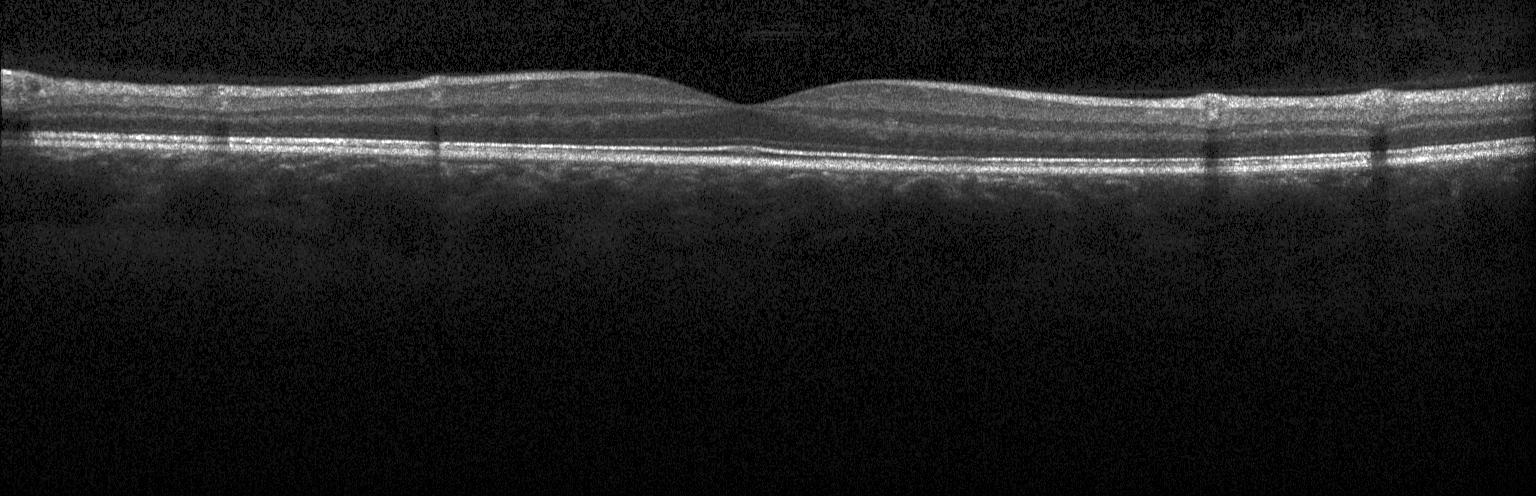 No CNV, no DME, and no drusen.